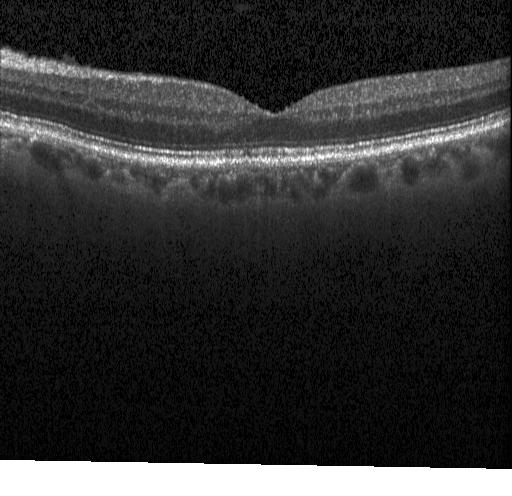

OCT B-scan showing no evidence of CNV, DME, or drusen.